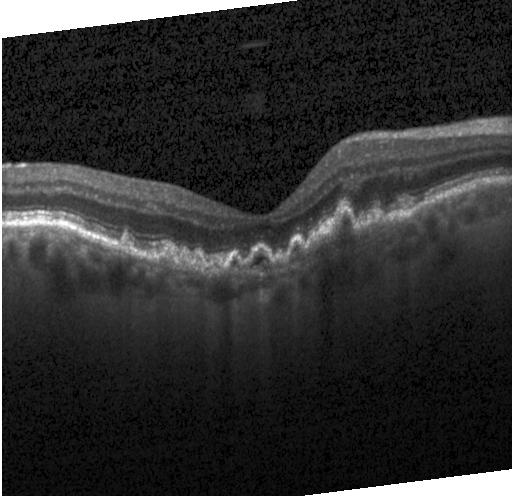 Horizontal scan through the fovea; retinal OCT B-scan; instrument: Heidelberg Spectralis; spectral-domain optical coherence tomography
Impression: choroidal neovascularization (CNV).